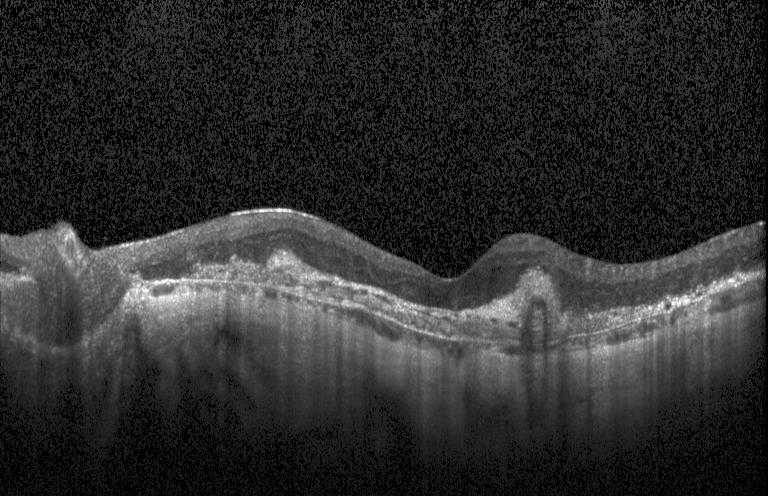
Retinal OCT B-scan — Choroidal neovascularization.